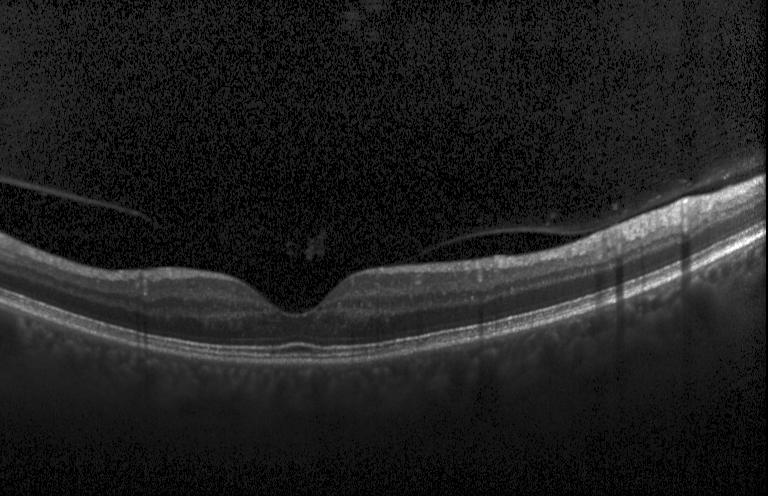
Acquired on a Heidelberg Spectralis. Spectral-domain optical coherence tomography. Through the macula. OCT line scan.
This B-scan demonstrates neither choroidal neovascularization, diabetic macular edema, nor drusen.